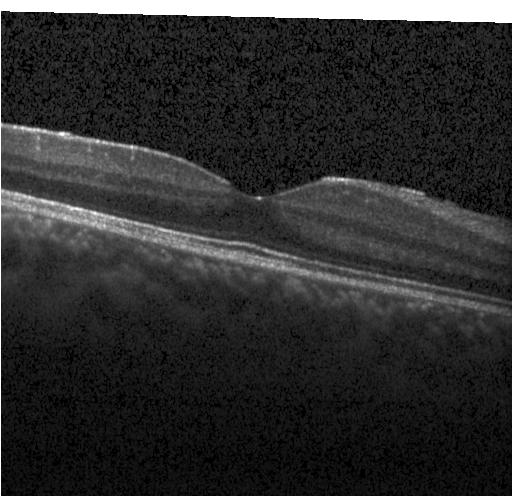 Retinal OCT cross-section — This B-scan demonstrates neither choroidal neovascularization, diabetic macular edema, nor drusen.